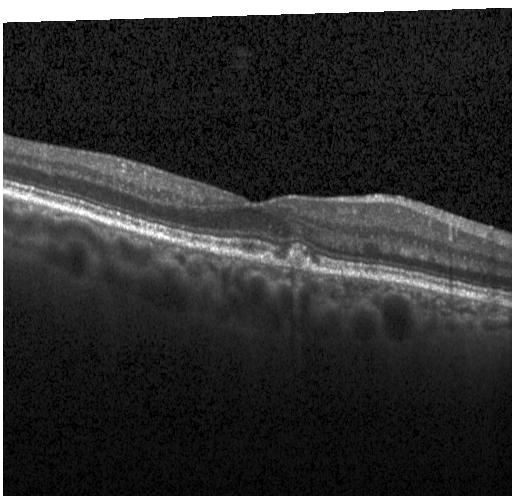

SD-OCT · OCT B-scan · instrument: Heidelberg Spectralis · fovea-centered
This B-scan demonstrates sub-RPE drusenoid deposits.